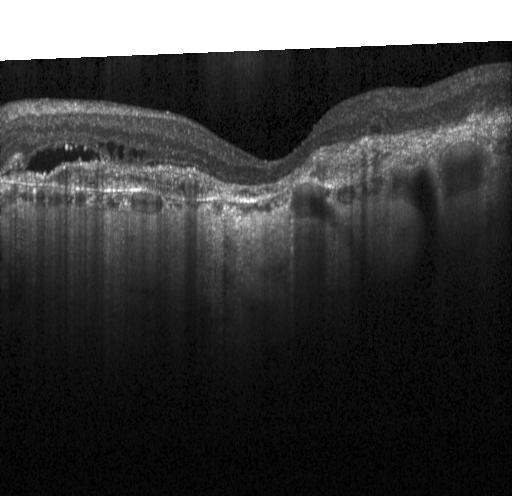

Spectral-domain optical coherence tomography. OCT B-scan.
A choroidal neovascular membrane.